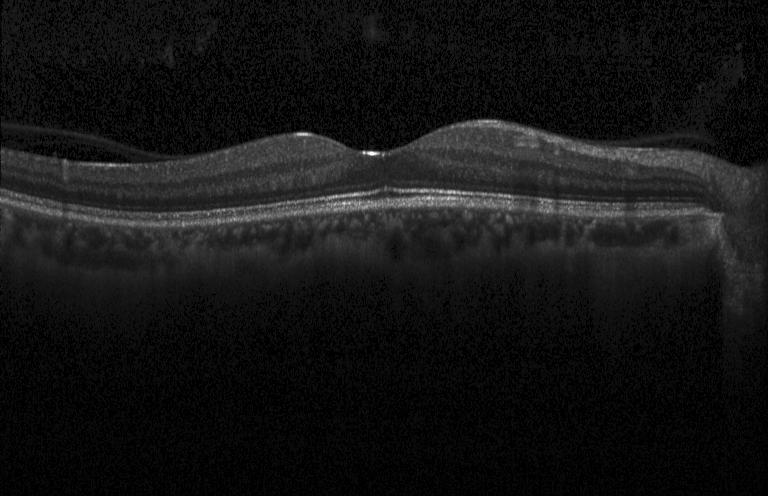
OCT line scan. Centered on the fovea — No choroidal neovascularization, diabetic macular edema, or drusen.